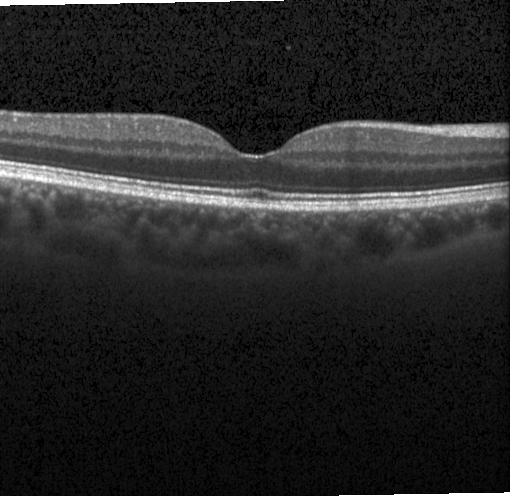
Dx: no CNV, no DME, and no drusen.